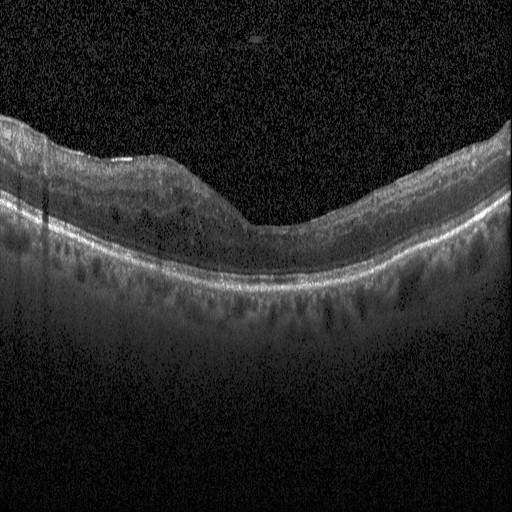

OCT line scan
Dx: DME.